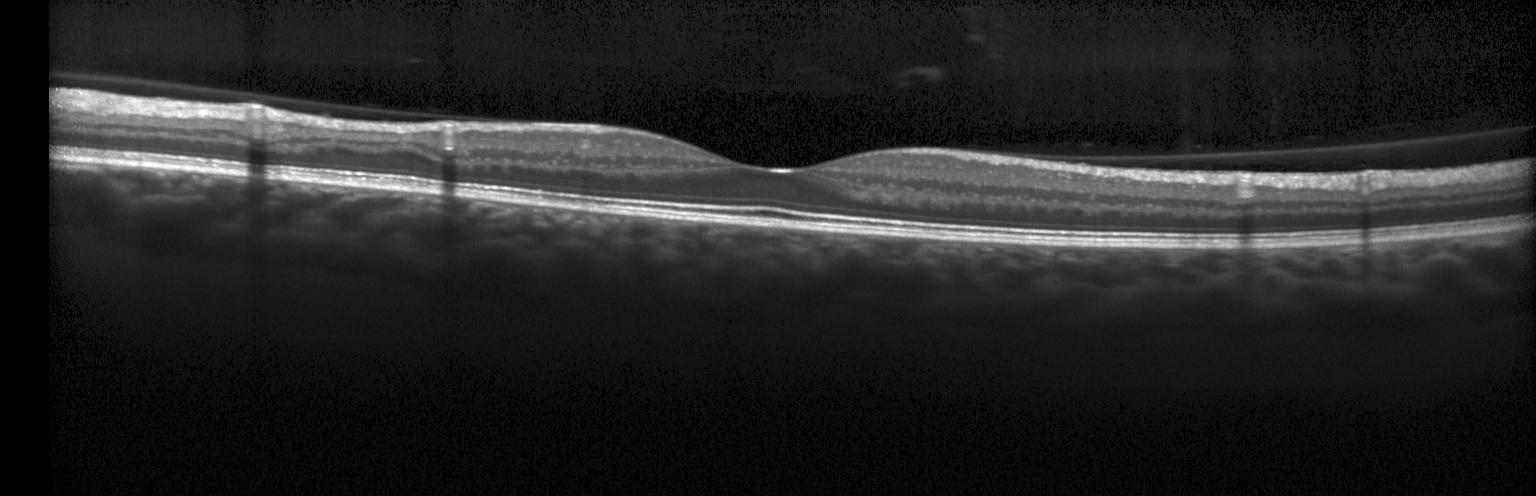
Retinal OCT cross-section.
Diagnosis: no evidence of choroidal neovascularization, diabetic macular edema, or drusen.